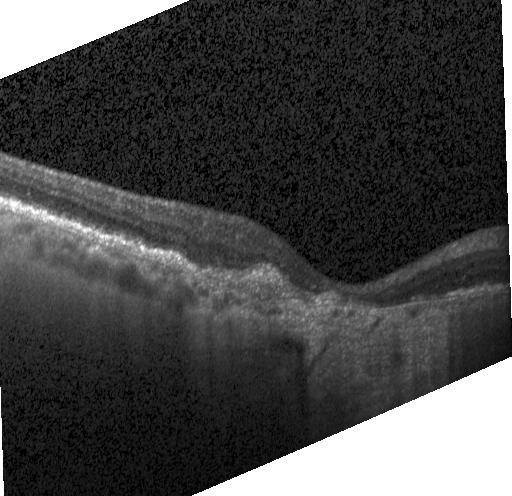
Impression: a choroidal neovascular membrane.